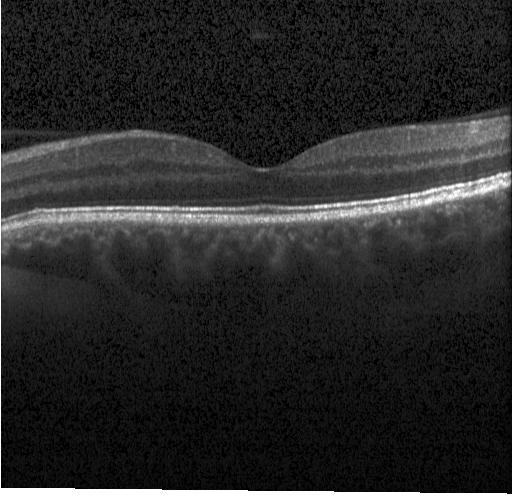

OCT line scan; centered on the fovea
Impression: neither choroidal neovascularization, diabetic macular edema, nor drusen.